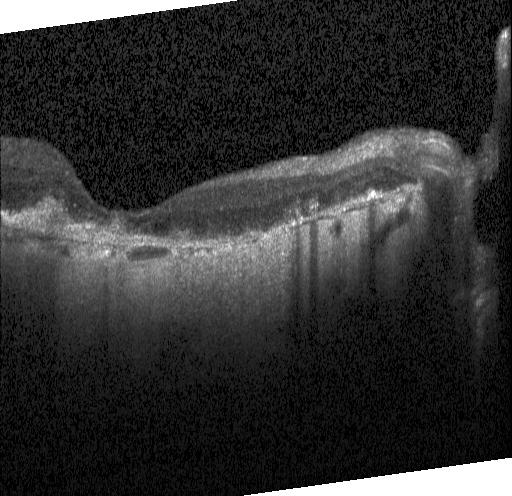
Fovea-centered; retinal OCT cross-section; SD-OCT. Finding: choroidal neovascularization.